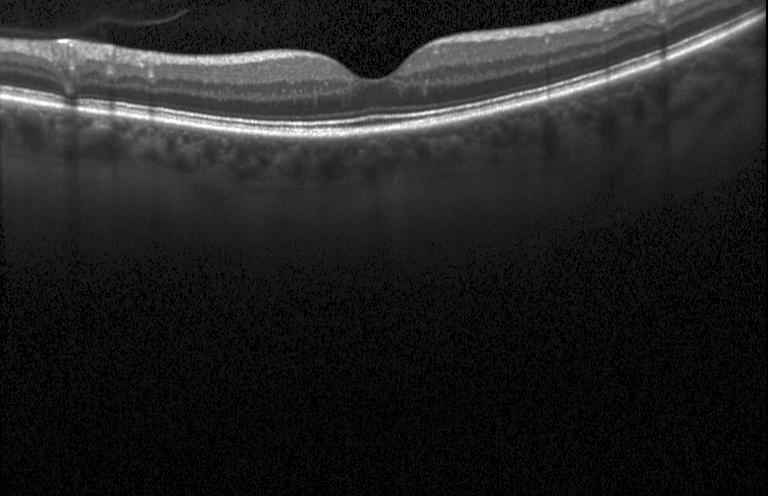 OCT scan showing neither CNV, DME, nor drusen.